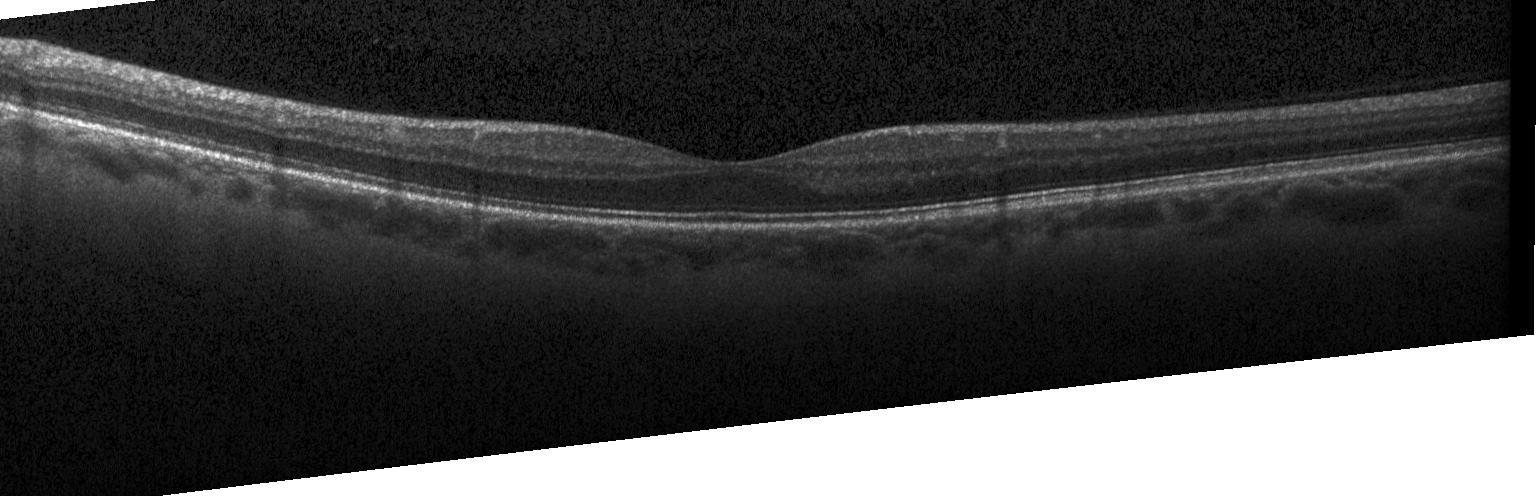
Retinal OCT cross-section · spectral-domain optical coherence tomography · fovea-centered. Dx: neither CNV, DME, nor drusen.